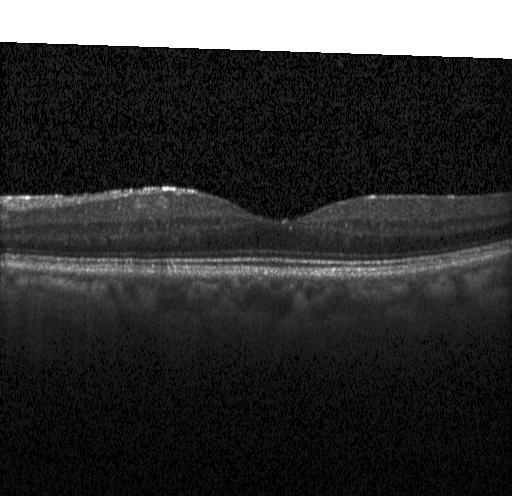
Centered on the fovea; OCT B-scan; Heidelberg Spectralis. The scan shows no CNV, DME, or drusen.